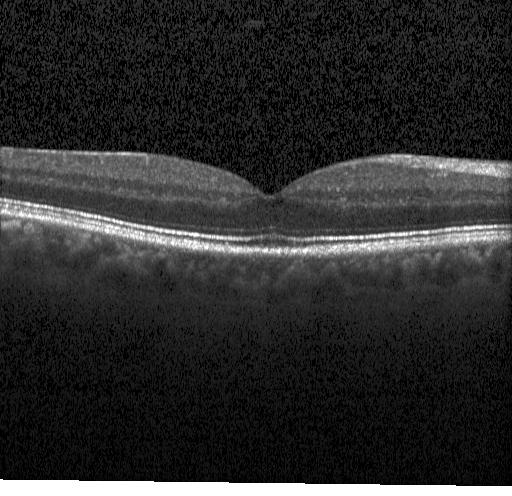

Macular OCT: no choroidal neovascularization, no diabetic macular edema, and no drusen.